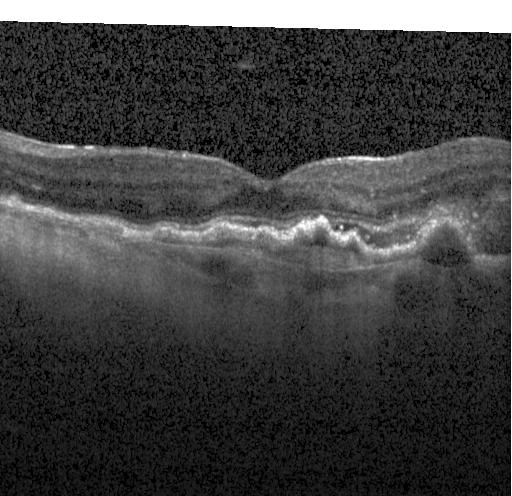

The scan shows choroidal neovascularization (CNV).